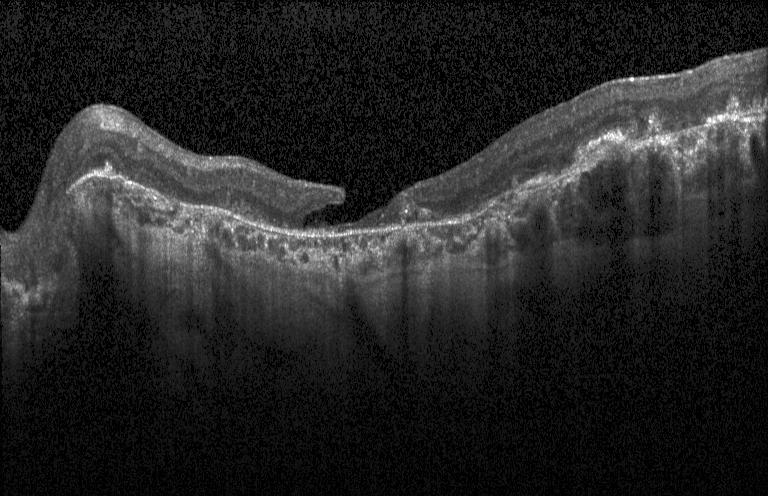 Macular OCT: choroidal neovascularization.